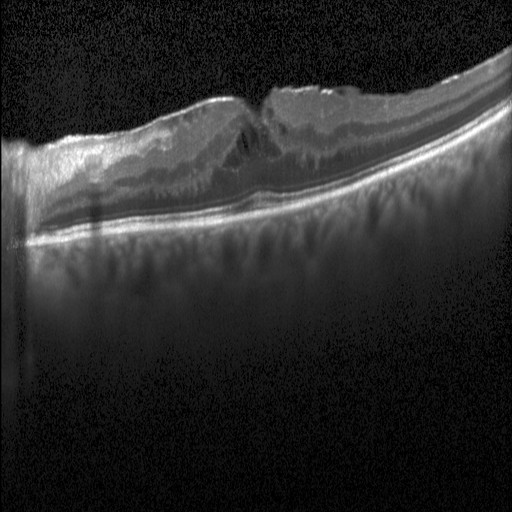

Optical coherence tomography B-scan
Diabetic macular edema.